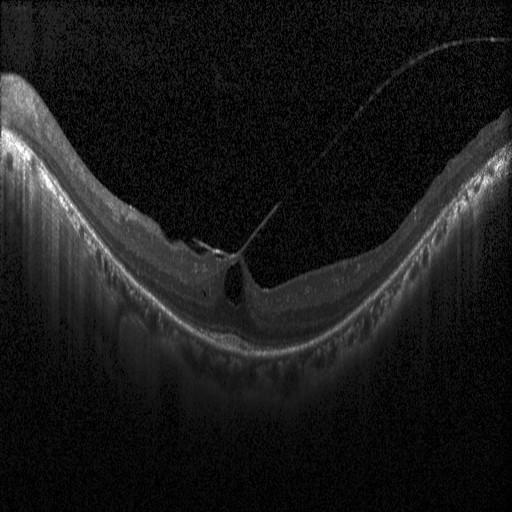

Horizontal scan through the fovea · retinal OCT B-scan. Impression: diabetic macular edema.